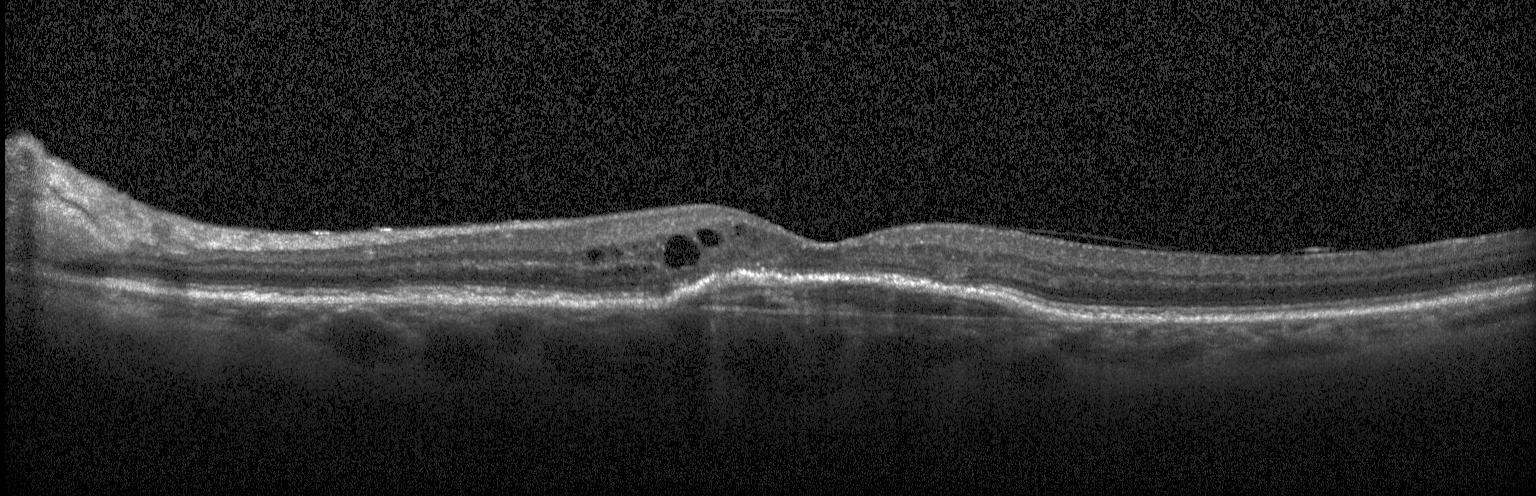
The scan shows a choroidal neovascular membrane.